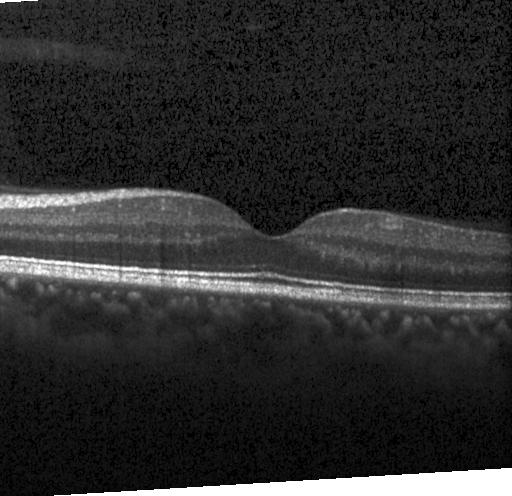
Finding: no evidence of choroidal neovascularization, diabetic macular edema, or drusen.